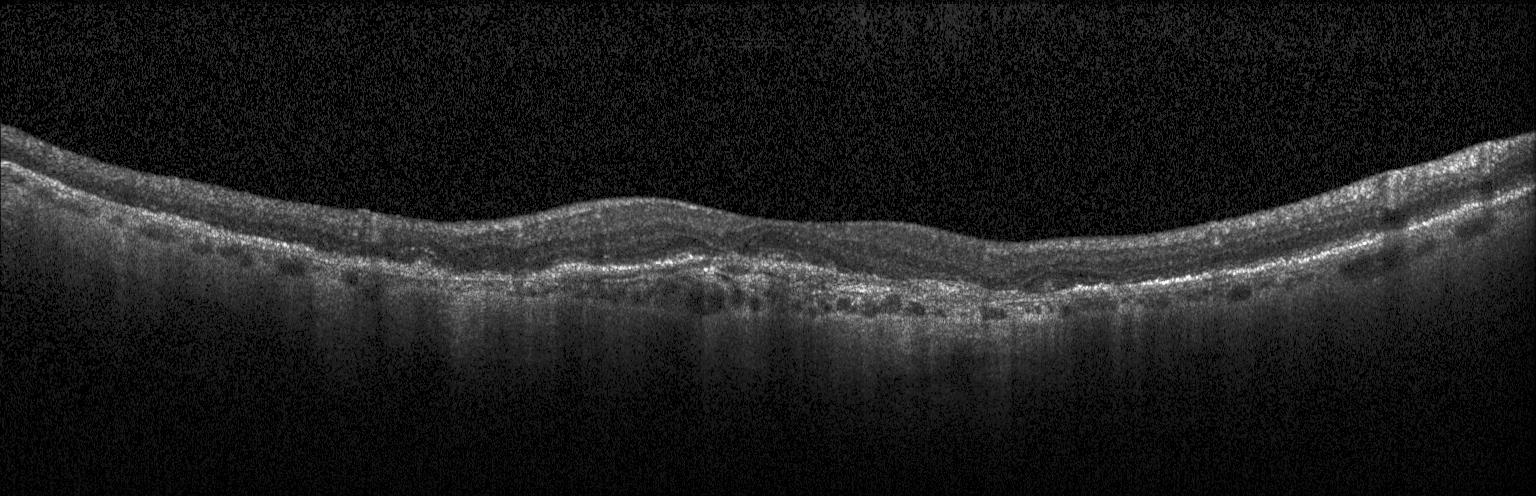 Acquired on a Heidelberg Spectralis. OCT B-scan. Horizontal scan through the fovea. Spectral-domain OCT
Macular OCT: choroidal neovascularization.